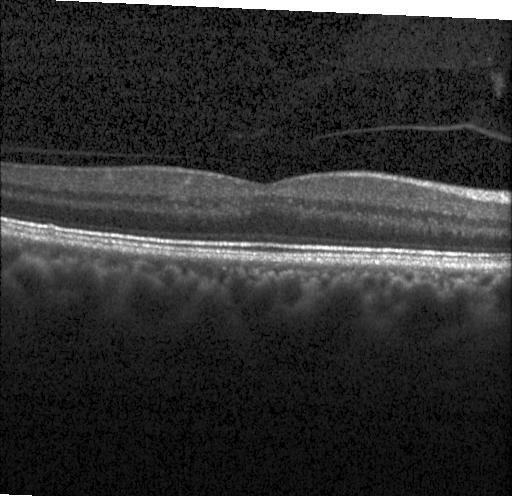 Heidelberg Spectralis OCT system, OCT B-scan. The scan shows neither choroidal neovascularization, diabetic macular edema, nor drusen.